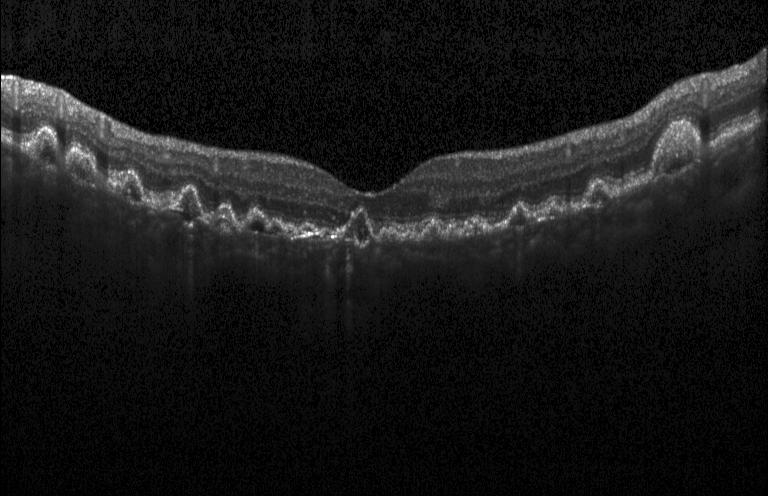
OCT B-scan.
A choroidal neovascular membrane.